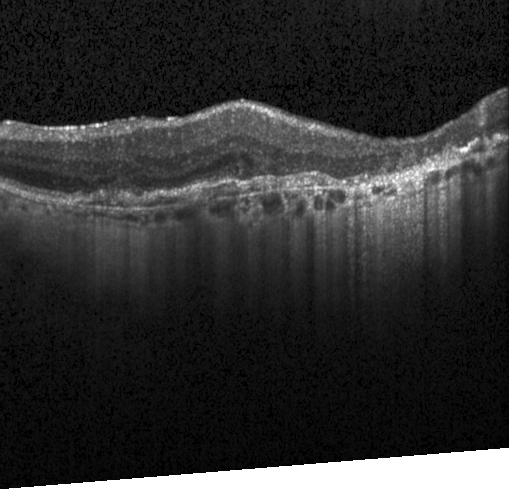
Centered on the fovea, optical coherence tomography B-scan, Heidelberg Spectralis — Macular OCT: choroidal neovascularization.